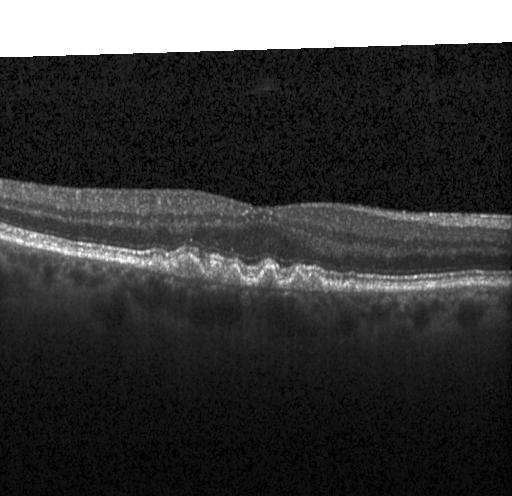 Macular OCT: sub-RPE drusenoid deposits.